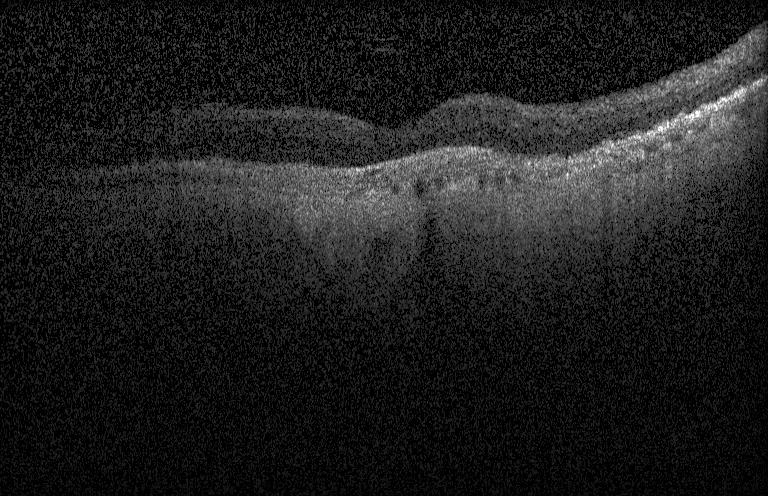
OCT scan showing a choroidal neovascular membrane.